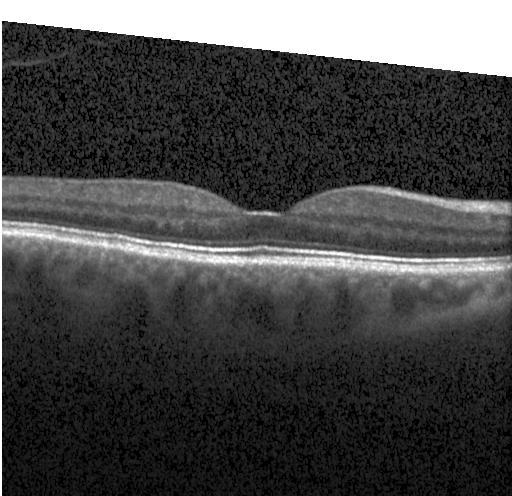

SD-OCT, instrument: Heidelberg Spectralis, optical coherence tomography scan
Dx: no evidence of choroidal neovascularization, diabetic macular edema, or drusen.